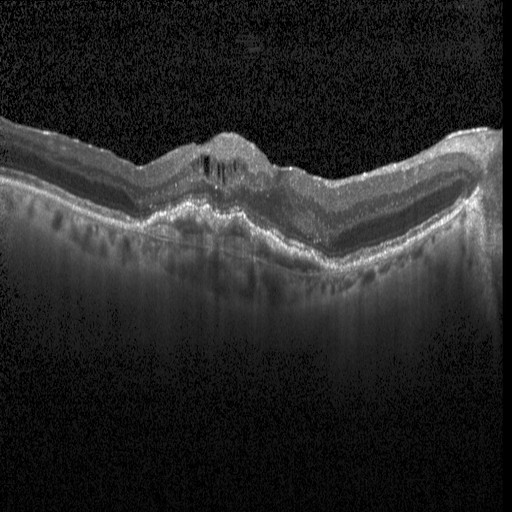 Macular OCT demonstrating DME.